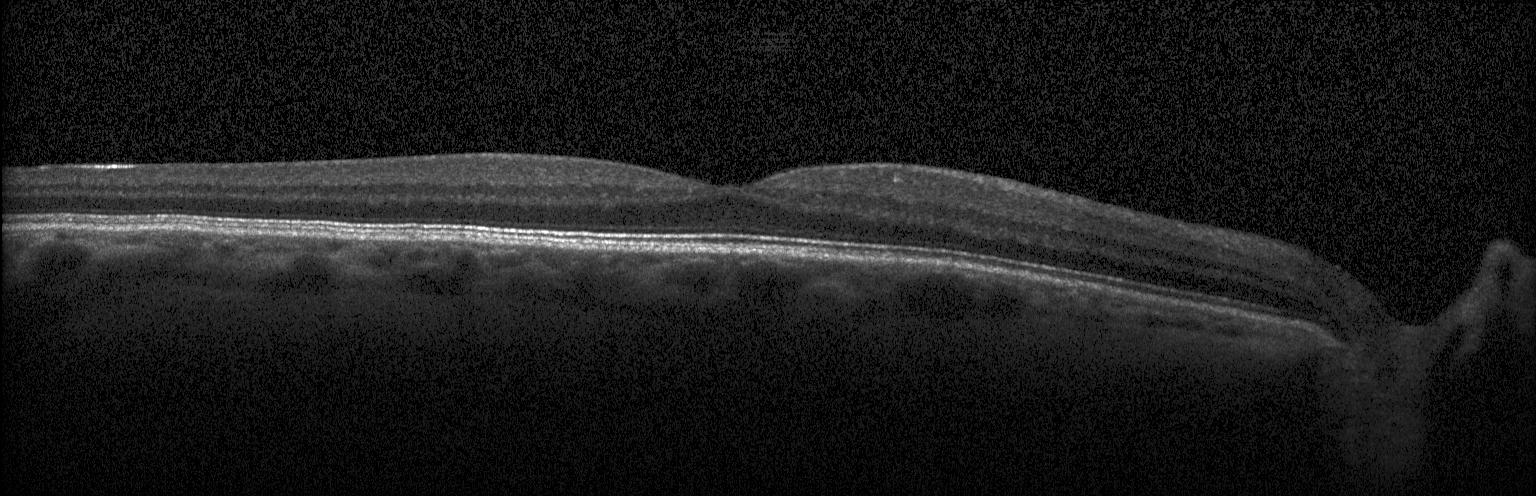 SD-OCT. OCT B-scan — Diagnosis: neither CNV, DME, nor drusen.